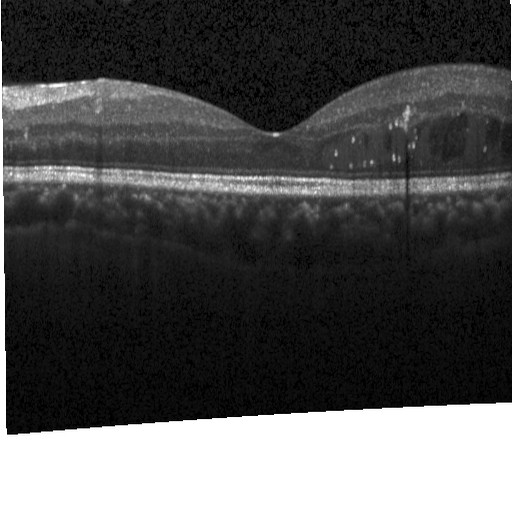 Heidelberg Spectralis OCT system · optical coherence tomography scan — Impression: diabetic macular edema.